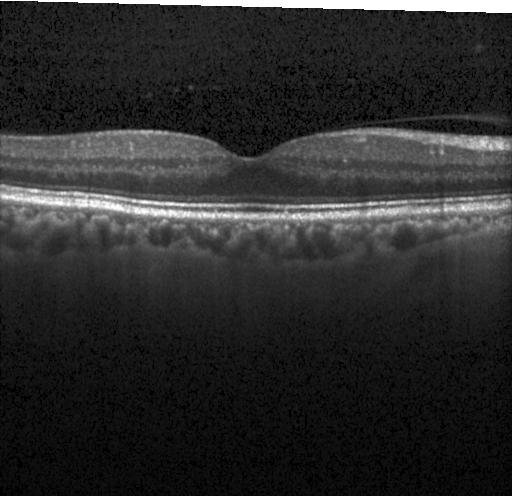 Spectral-domain optical coherence tomography · fovea-centered · OCT B-scan — The scan shows no evidence of choroidal neovascularization, diabetic macular edema, or drusen.